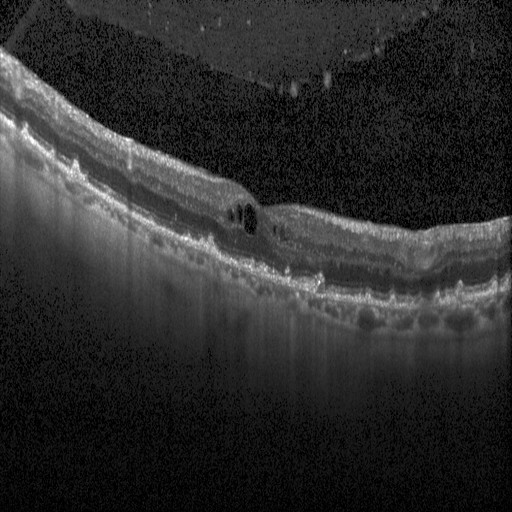
Macular OCT: diabetic macular edema (DME).